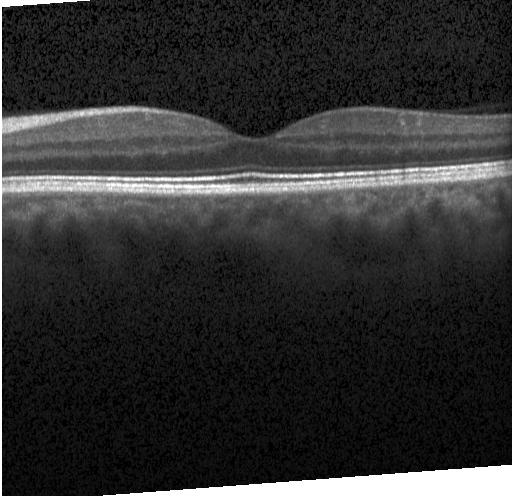
Retinal OCT B-scan.
Finding: no evidence of CNV, DME, or drusen.